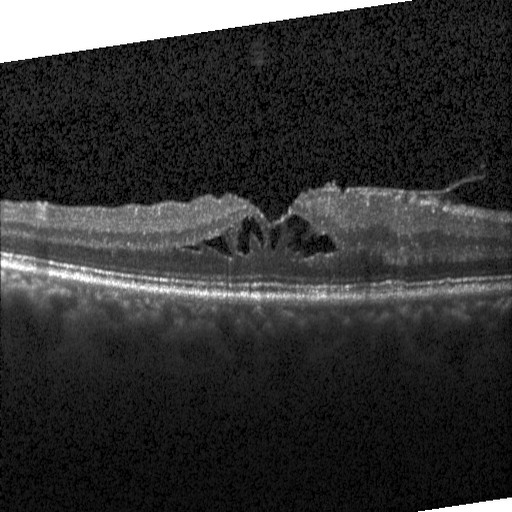 OCT finding: DME.